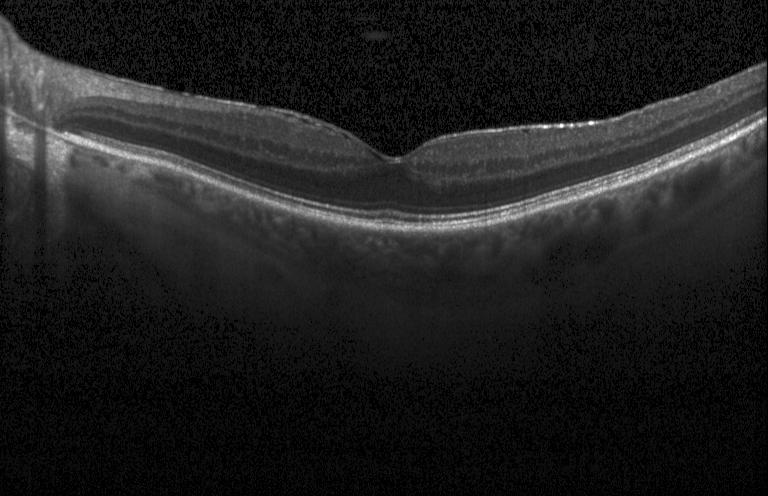

Fovea-centered, Heidelberg Spectralis OCT system, optical coherence tomography scan, spectral-domain optical coherence tomography
This B-scan demonstrates no choroidal neovascularization, diabetic macular edema, or drusen.